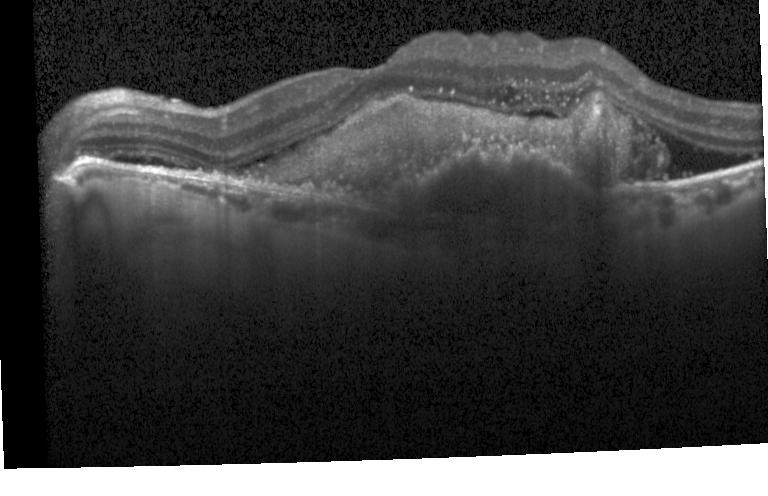
Macular OCT: CNV.